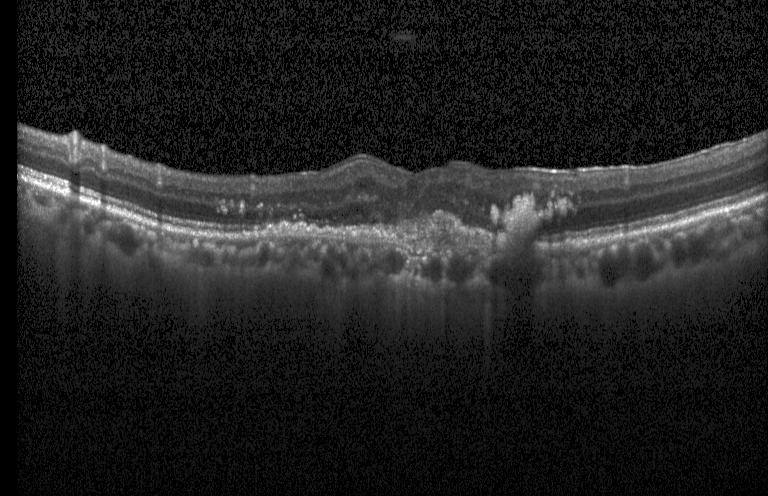 Spectral-domain OCT B-scan: a choroidal neovascular membrane.